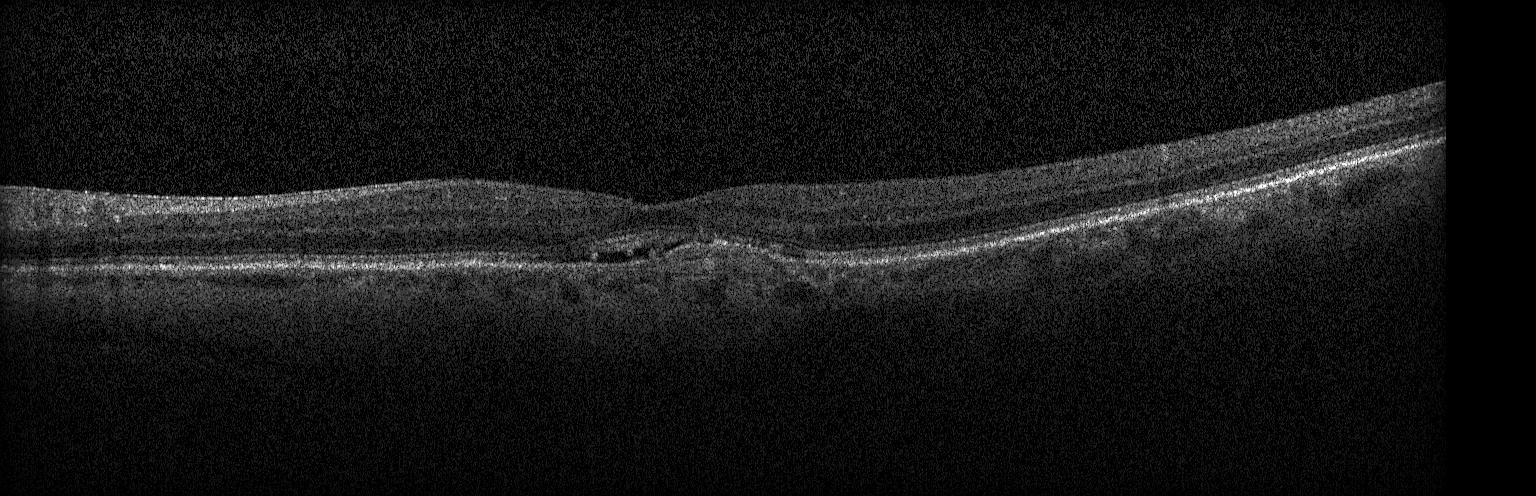 Spectral-domain optical coherence tomography · retinal OCT B-scan · fovea-centered · Heidelberg Spectralis.
The scan shows choroidal neovascularization.